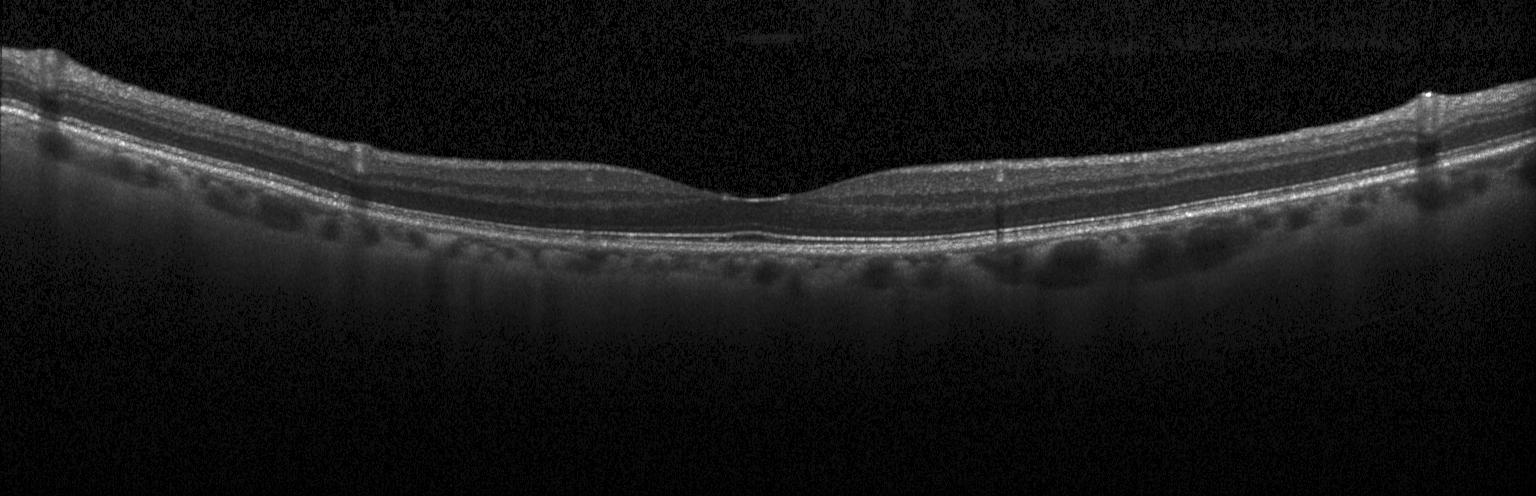 OCT line scan — The scan shows no choroidal neovascularization, no diabetic macular edema, and no drusen.